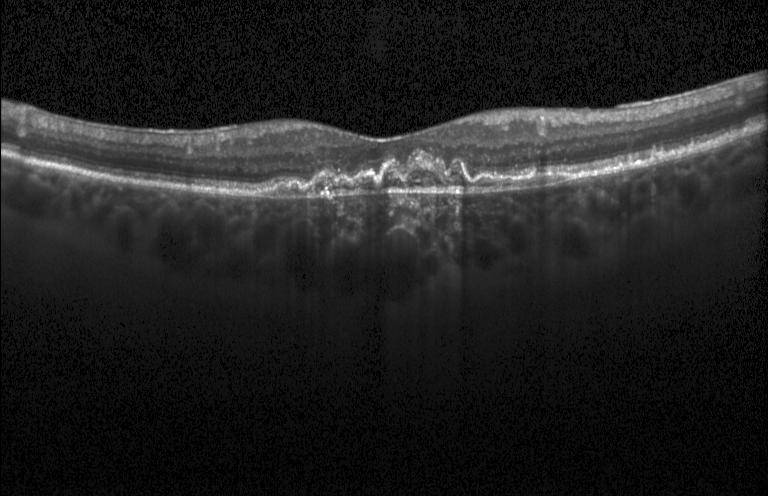 Retinal OCT cross-section showing a choroidal neovascular membrane.